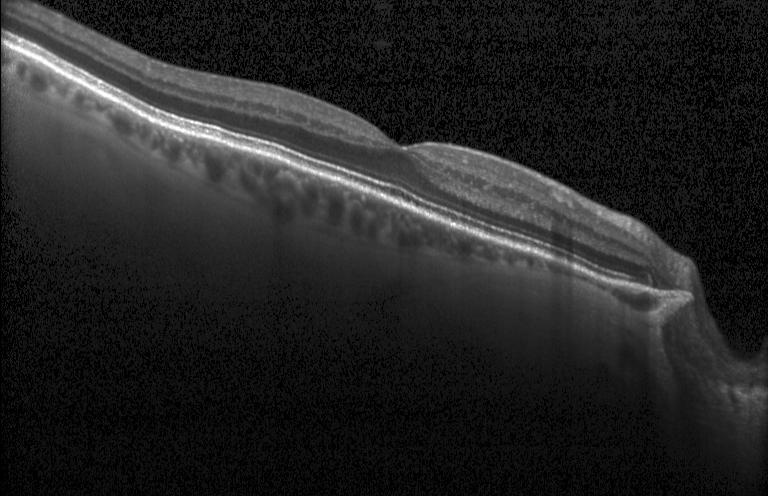 Heidelberg Spectralis OCT system, through the macula, optical coherence tomography B-scan
Finding: no choroidal neovascularization, diabetic macular edema, or drusen.